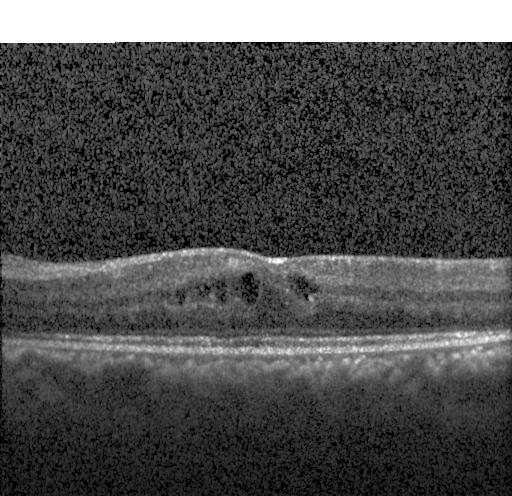 Diagnosis: DME.